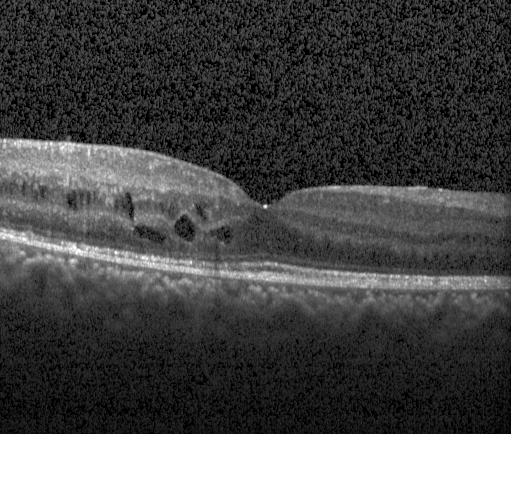 Horizontal scan through the fovea · instrument: Heidelberg Spectralis · optical coherence tomography scan · spectral-domain OCT
Impression: diabetic macular edema (DME).